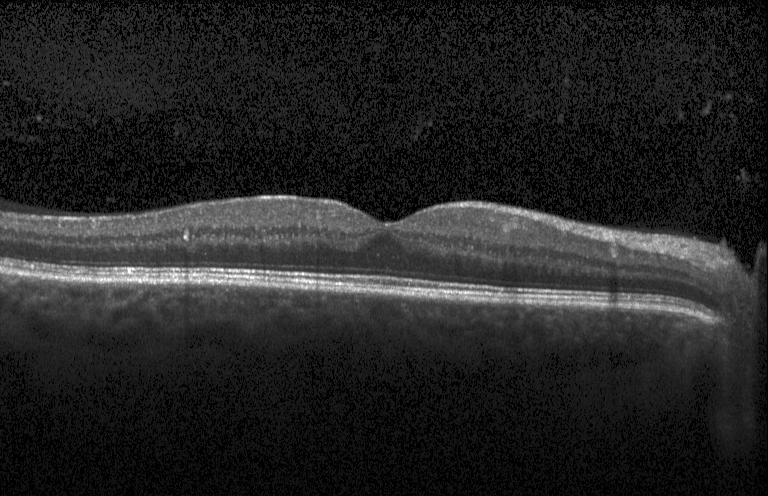

Instrument: Heidelberg Spectralis, spectral-domain optical coherence tomography, OCT B-scan, centered on the fovea.
Finding: no evidence of choroidal neovascularization, diabetic macular edema, or drusen.